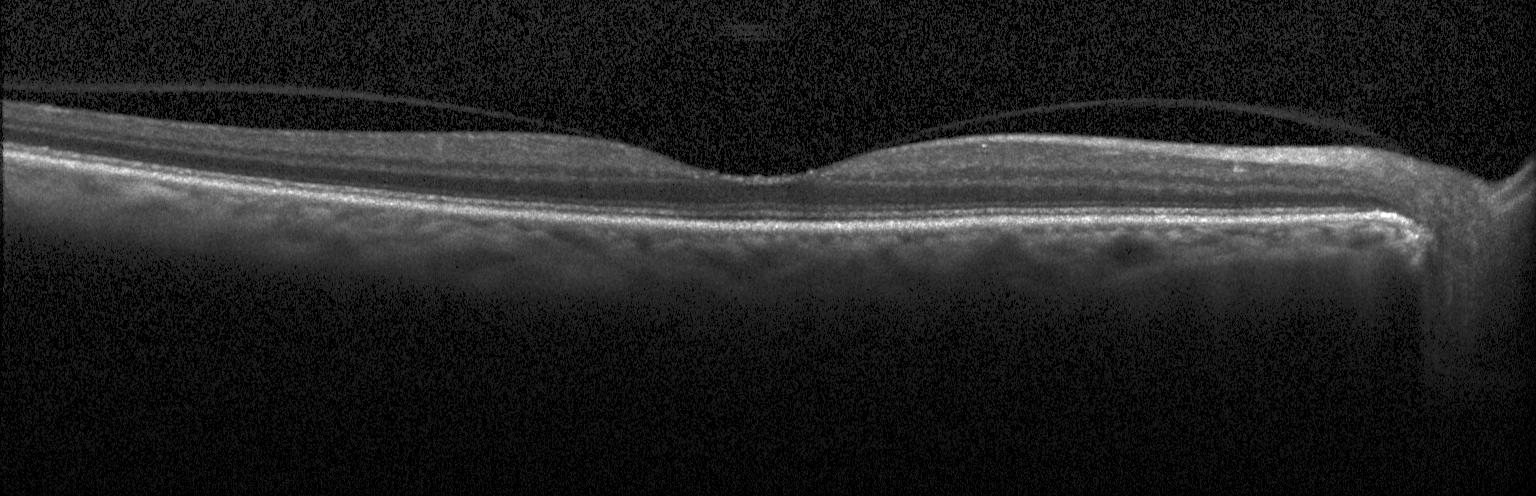
The scan shows no CNV, DME, or drusen.